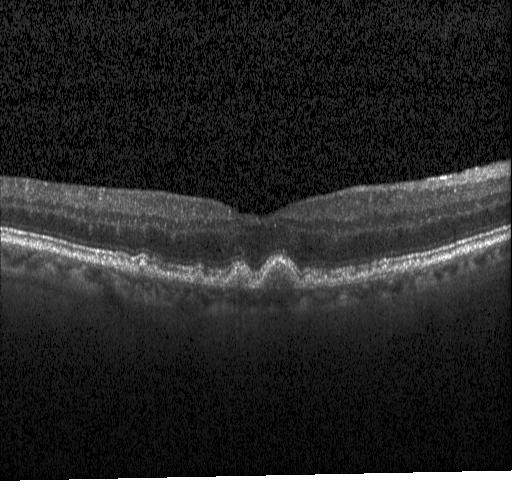
OCT B-scan
Finding: drusen.